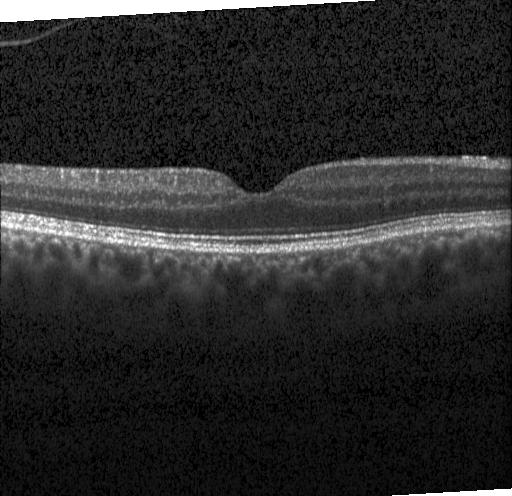
OCT line scan — This B-scan demonstrates neither choroidal neovascularization, diabetic macular edema, nor drusen.